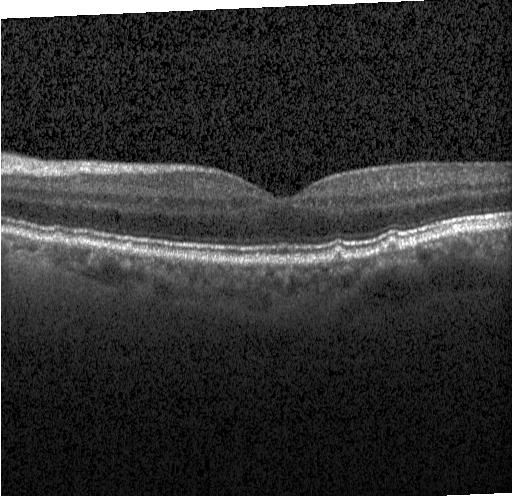
Retinal OCT cross-section, macular scan. Impression: drusen.